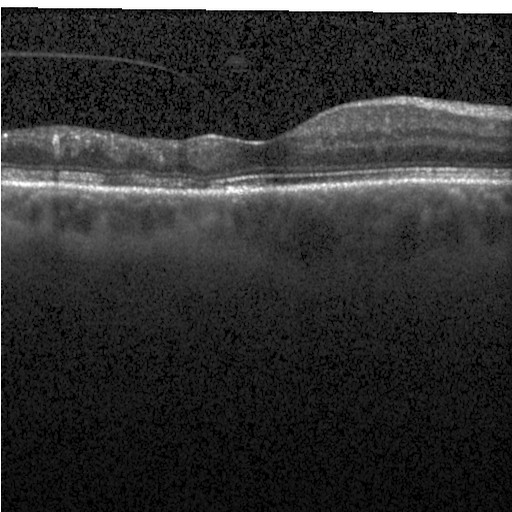

Macular scan. Retinal OCT B-scan. Instrument: Heidelberg Spectralis — The scan shows DME.